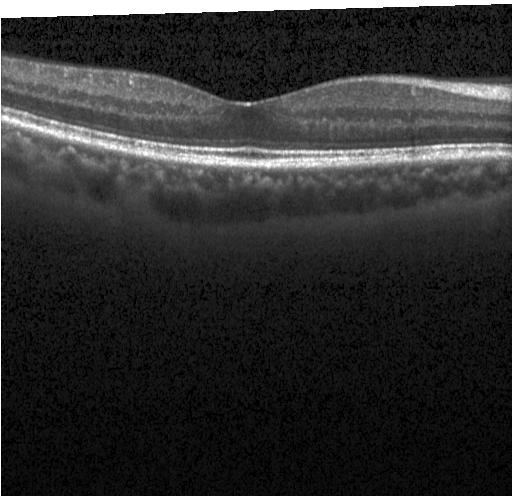

SD-OCT · OCT B-scan — Diagnosis: no choroidal neovascularization, no diabetic macular edema, and no drusen.